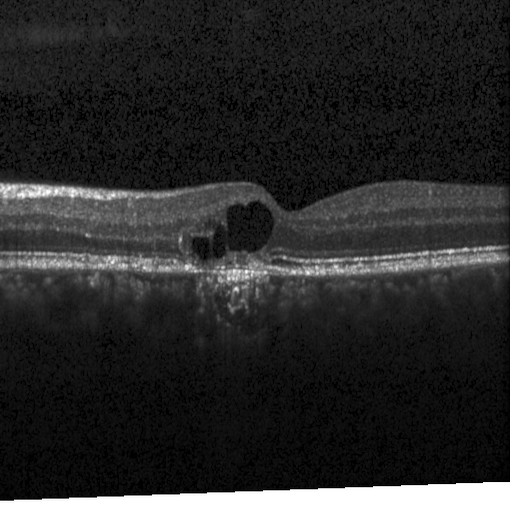
This B-scan demonstrates DME.